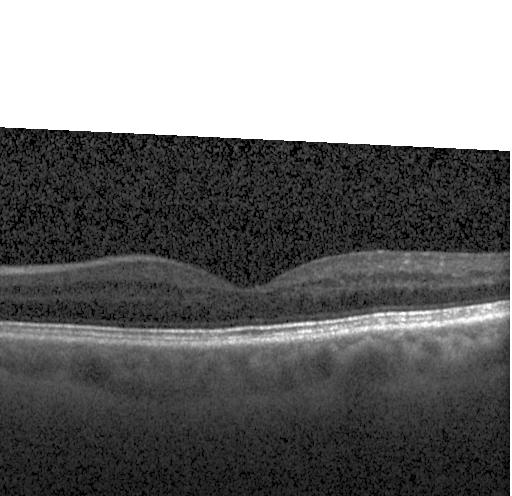 The scan shows no choroidal neovascularization, no diabetic macular edema, and no drusen.